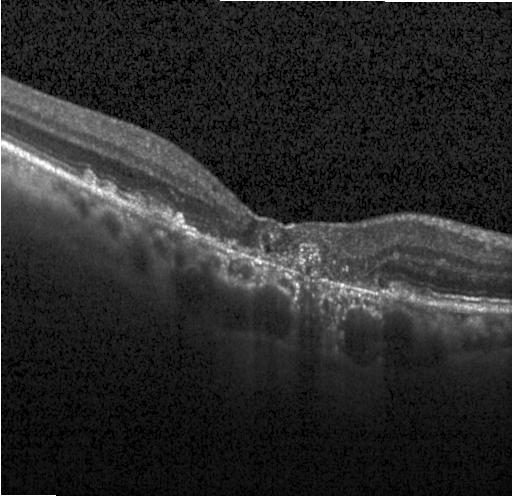
OCT line scan.
The scan shows a choroidal neovascular membrane.